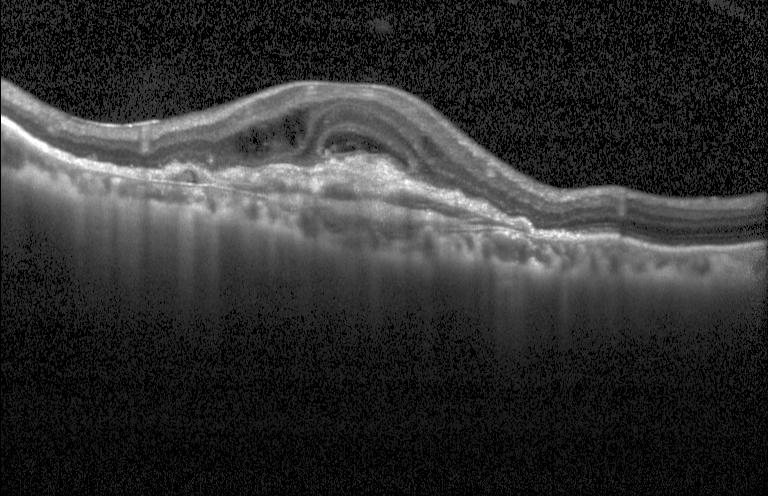
Retinal OCT cross-section showing choroidal neovascularization (CNV).